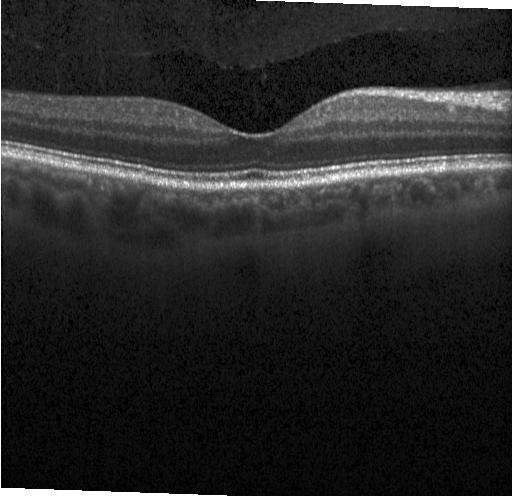
No choroidal neovascularization, diabetic macular edema, or drusen.